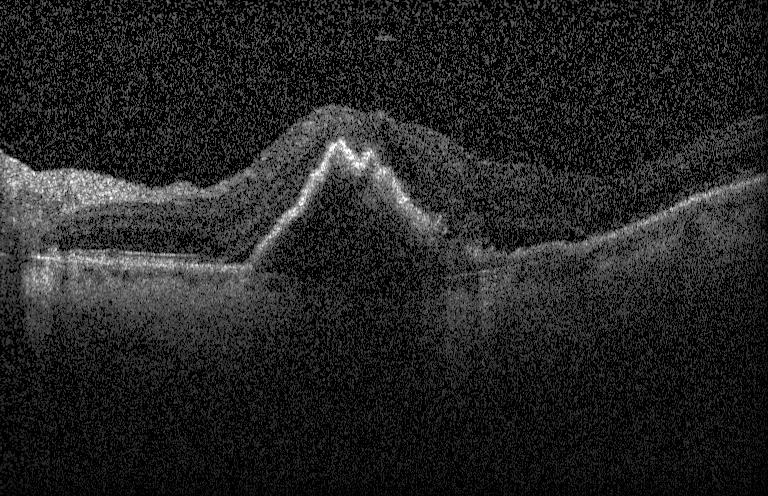

Retinal OCT B-scan, Heidelberg Spectralis OCT system.
Choroidal neovascularization (CNV).